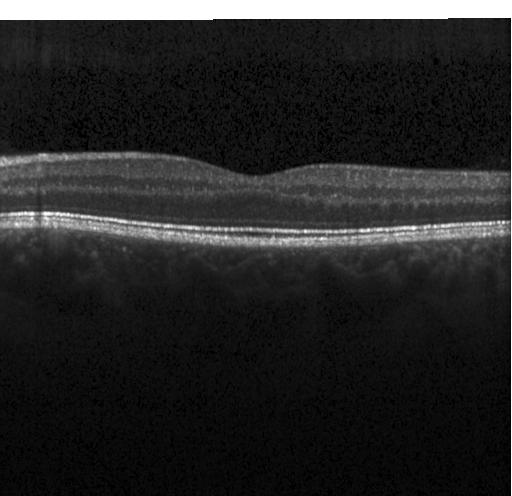

SD-OCT, retinal OCT cross-section.
Dx: no choroidal neovascularization, no diabetic macular edema, and no drusen.